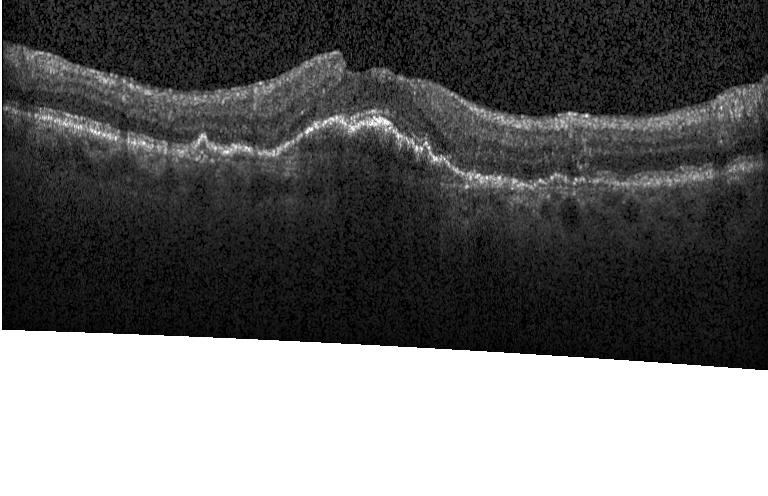

Assessment: CNV.